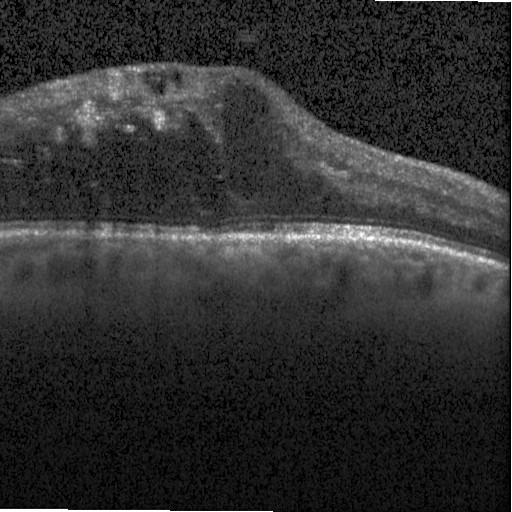
Macular OCT: diabetic macular edema.